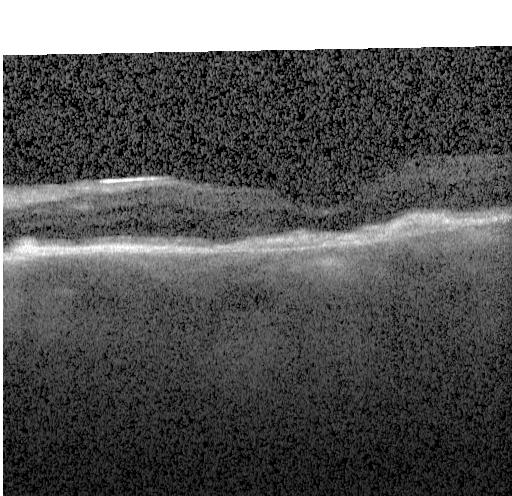

Impression: choroidal neovascularization.